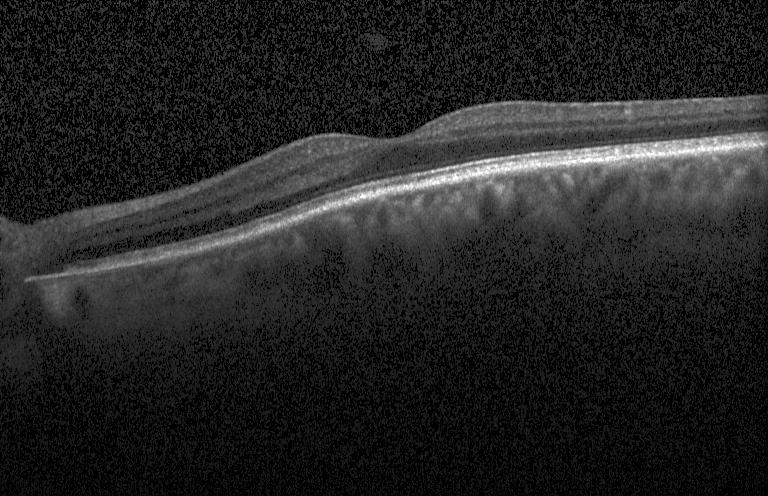

Fovea-centered; optical coherence tomography B-scan; spectral-domain OCT; instrument: Heidelberg Spectralis
Assessment: no choroidal neovascularization, no diabetic macular edema, and no drusen.